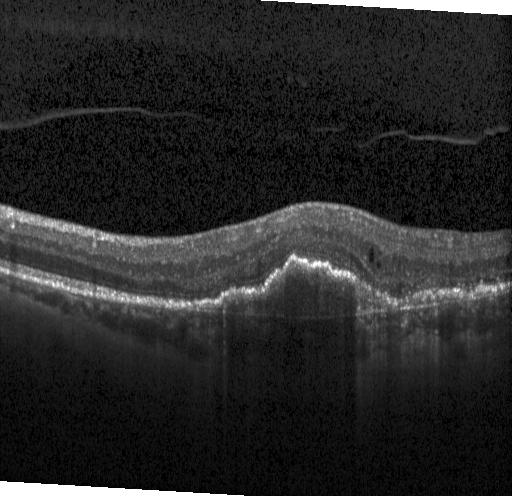

Macular scan; optical coherence tomography B-scan.
Impression: choroidal neovascularization.